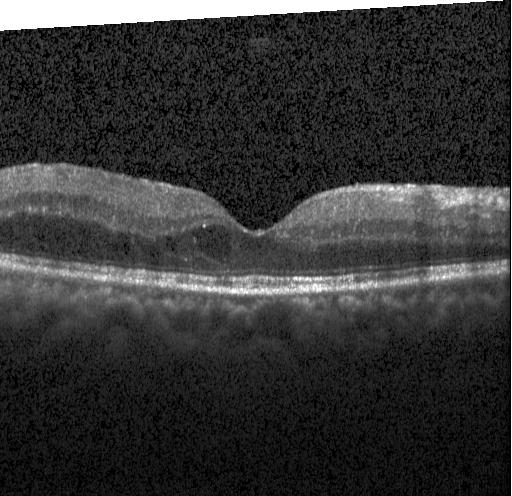

Diagnosis: DME.